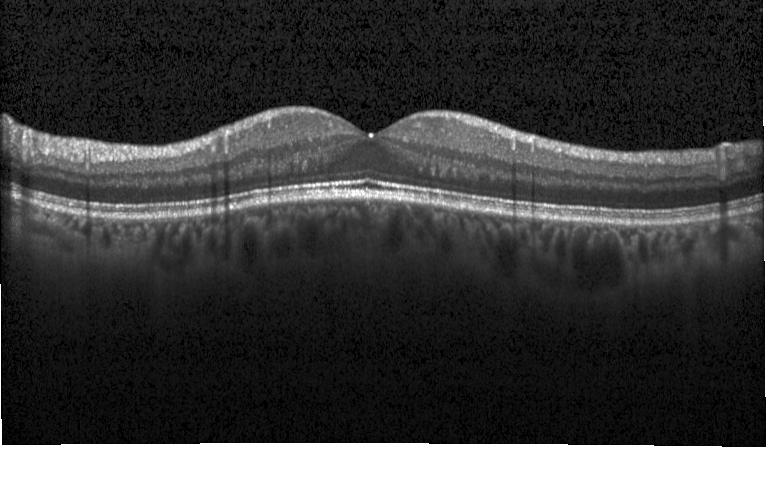

Optical coherence tomography scan.
No evidence of CNV, DME, or drusen.